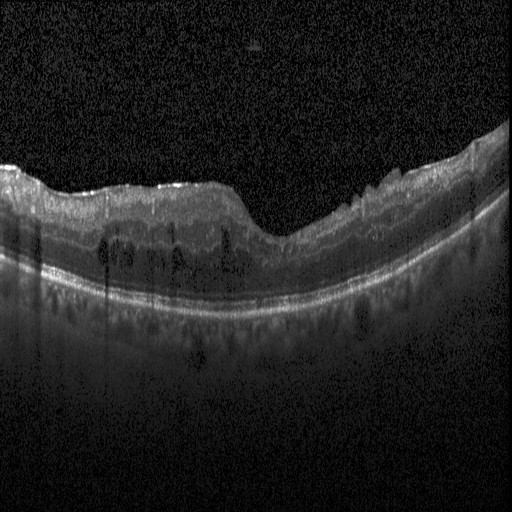

Optical coherence tomography B-scan.
Macular OCT: diabetic macular edema (DME).